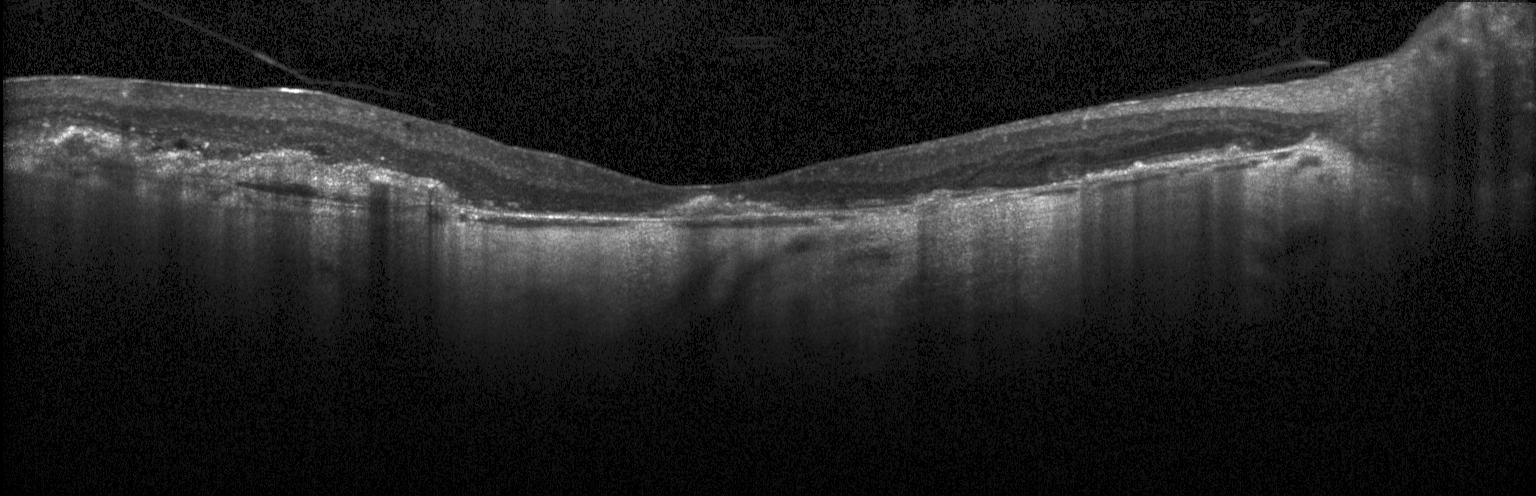
Dx: CNV.